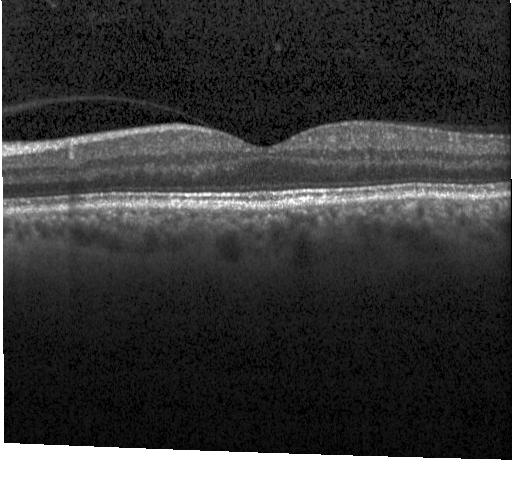 OCT line scan, acquired on a Heidelberg Spectralis, spectral-domain OCT — Dx: no evidence of choroidal neovascularization, diabetic macular edema, or drusen.